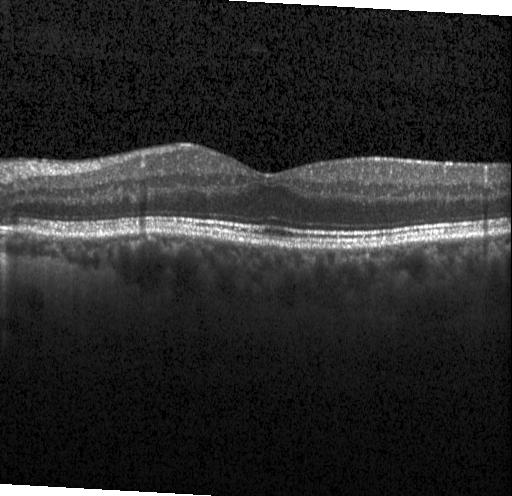 Optical coherence tomography B-scan.
OCT finding: neither choroidal neovascularization, diabetic macular edema, nor drusen.